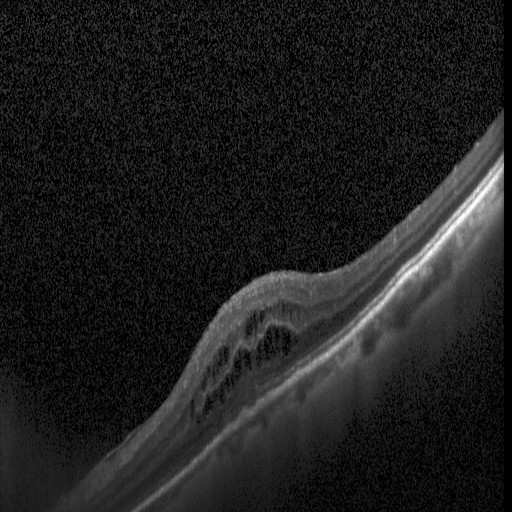
Acquired on a Heidelberg Spectralis; optical coherence tomography scan. Impression: DME.